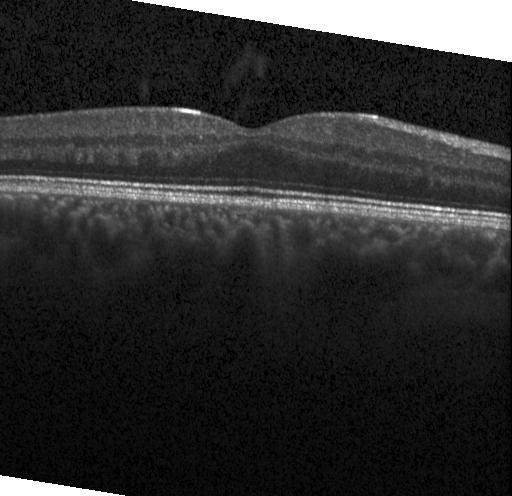
Horizontal scan through the fovea · optical coherence tomography B-scan · acquired on a Heidelberg Spectralis · spectral-domain optical coherence tomography
Impression: neither CNV, DME, nor drusen.